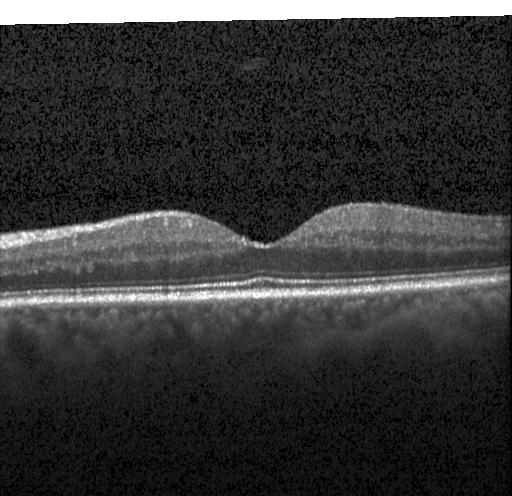

OCT B-scan; Heidelberg Spectralis; spectral-domain optical coherence tomography.
Impression: no choroidal neovascularization, no diabetic macular edema, and no drusen.